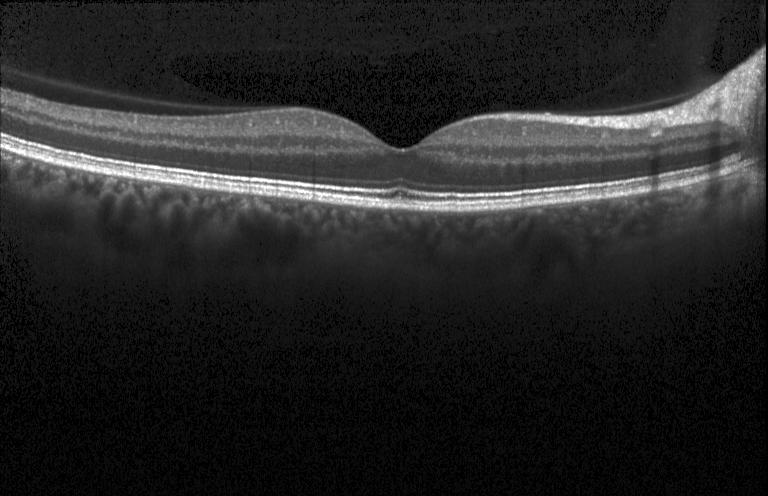 Retinal OCT B-scan.
Diagnosis: no evidence of CNV, DME, or drusen.